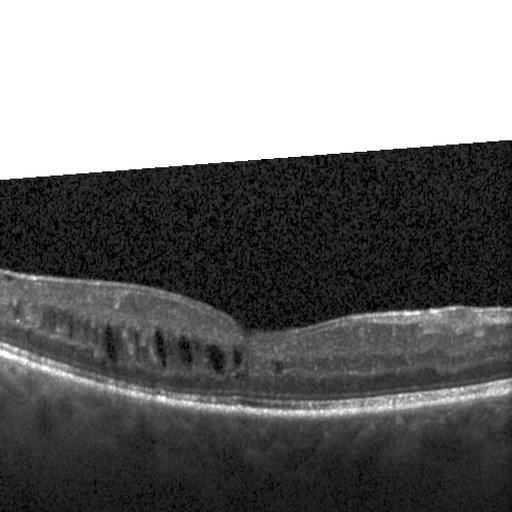
Heidelberg Spectralis. Centered on the fovea. Retinal OCT B-scan. Spectral-domain optical coherence tomography — Diagnosis: DME.